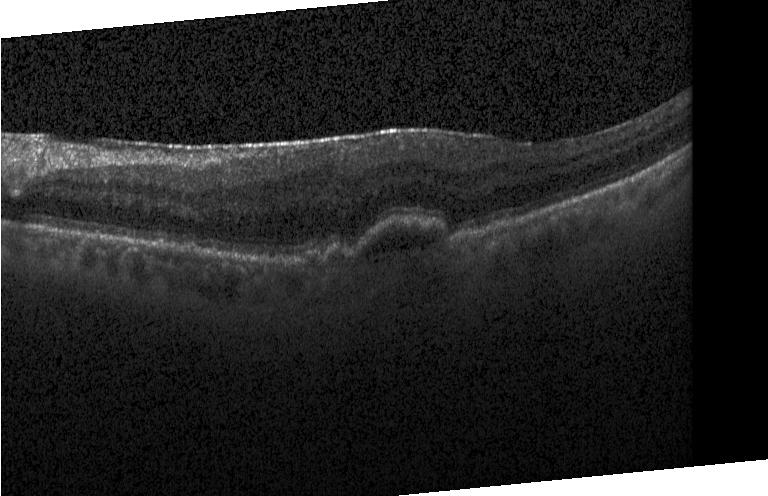

Optical coherence tomography B-scan
Impression: choroidal neovascularization.